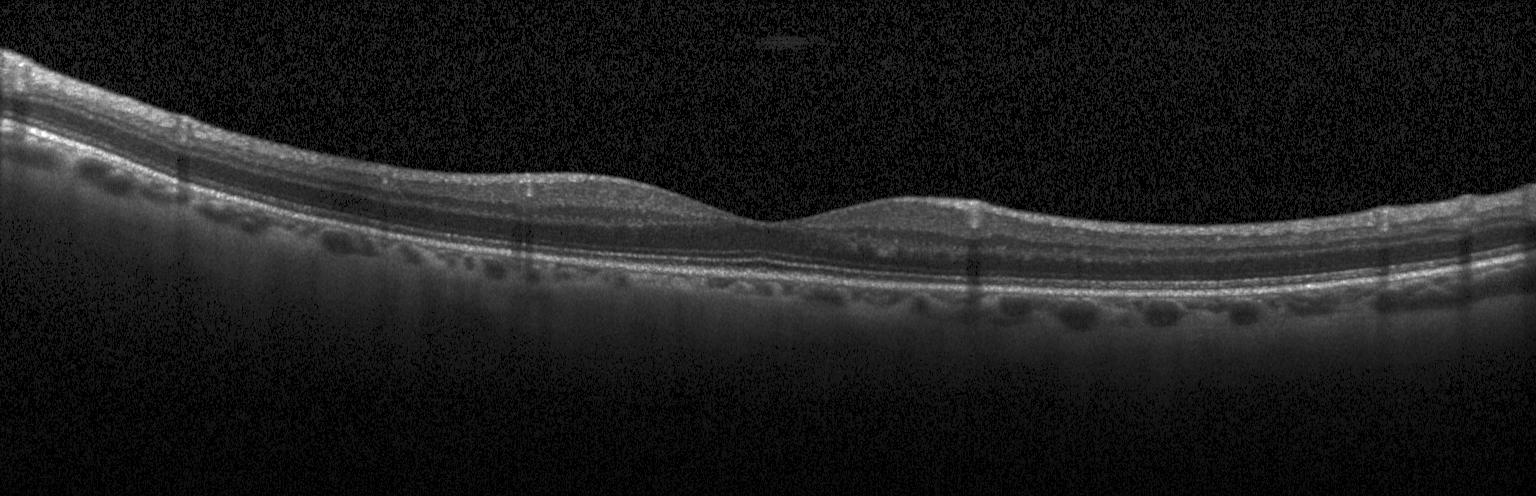
The scan shows no CNV, DME, or drusen.